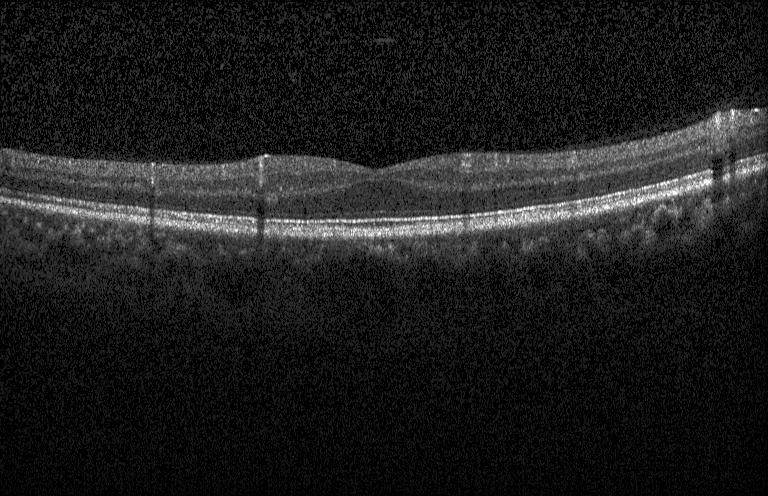 Impression: no CNV, no DME, and no drusen.